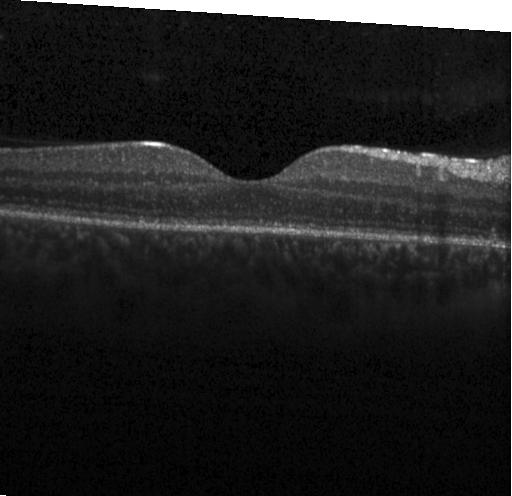

Impression: neither CNV, DME, nor drusen.